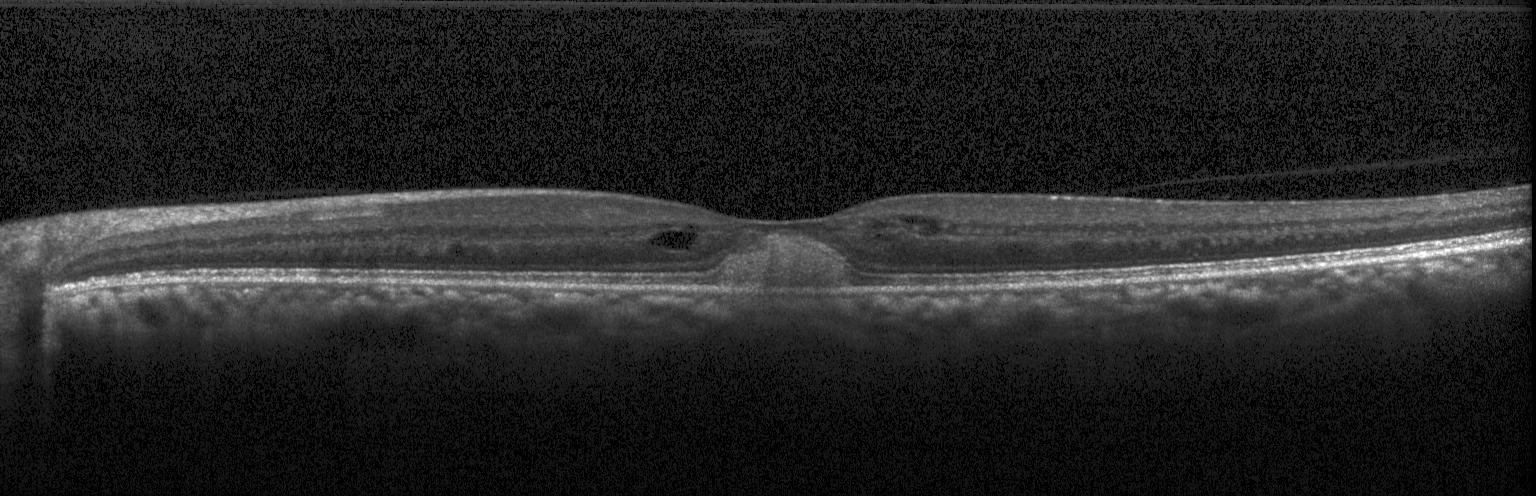 Macular OCT: a choroidal neovascular membrane.